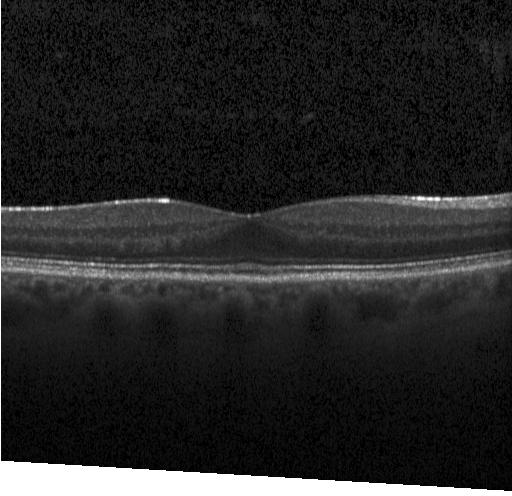
OCT B-scan · horizontal scan through the fovea · spectral-domain OCT
No evidence of choroidal neovascularization, diabetic macular edema, or drusen.